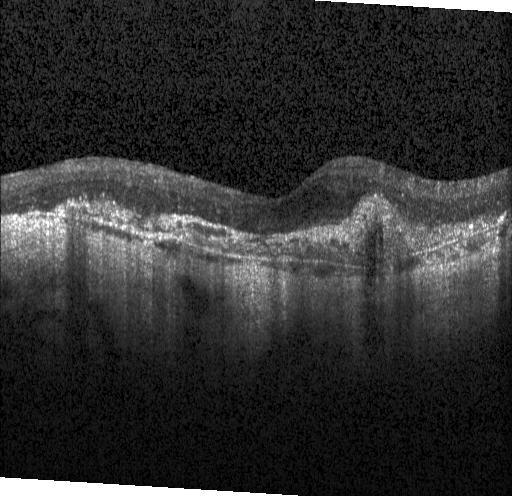 Retinal OCT B-scan · acquired on a Heidelberg Spectralis · fovea-centered · SD-OCT — OCT finding: CNV.